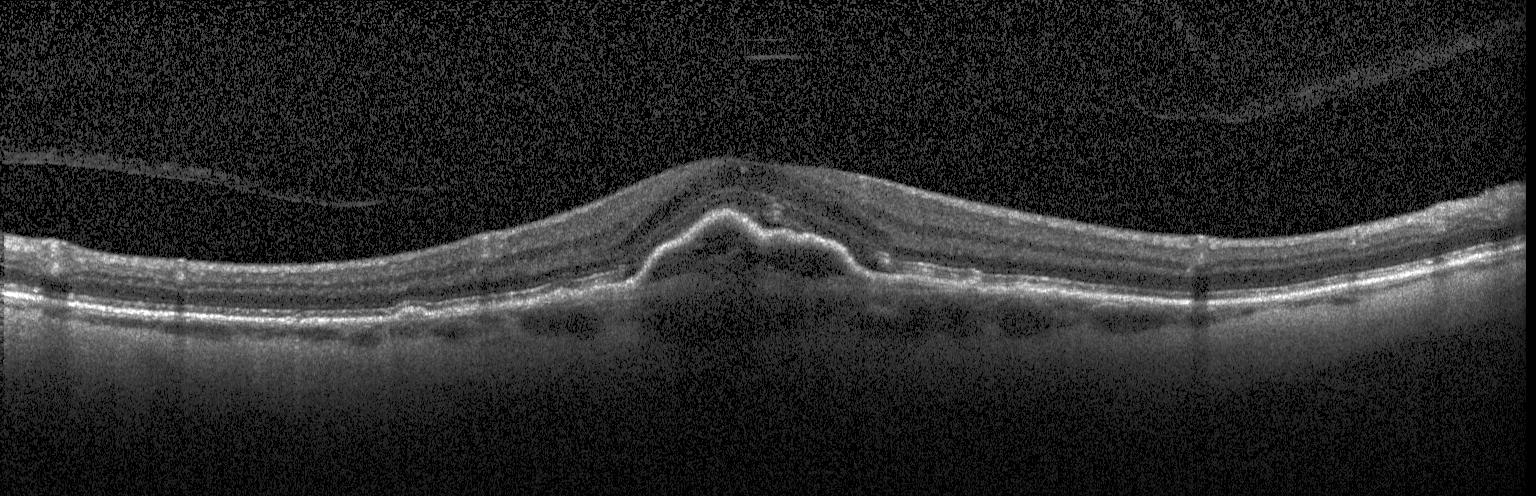

Retinal OCT cross-section showing a choroidal neovascular membrane.